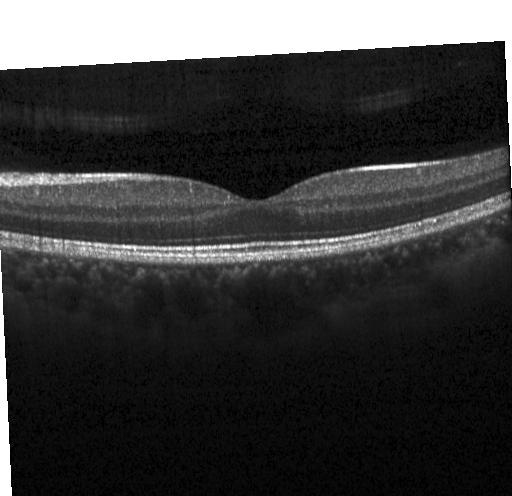

OCT B-scan; Heidelberg Spectralis OCT system; spectral-domain optical coherence tomography. Finding: neither choroidal neovascularization, diabetic macular edema, nor drusen.